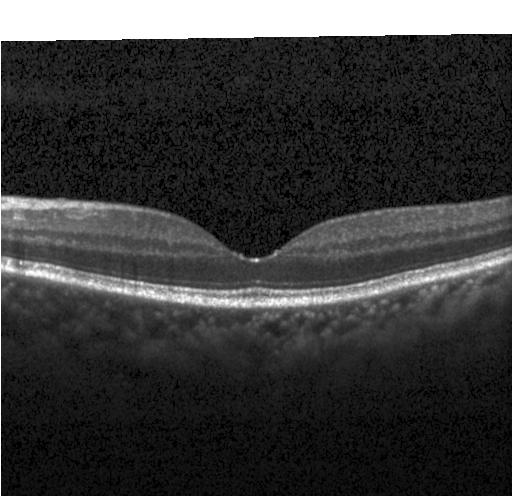
OCT line scan — Finding: no choroidal neovascularization, diabetic macular edema, or drusen.